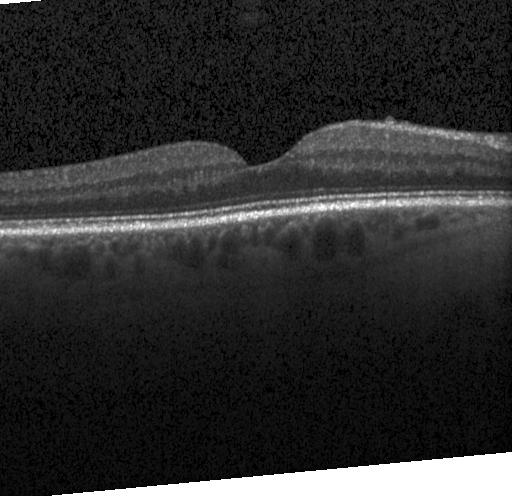 Spectral-domain optical coherence tomography · acquired on a Heidelberg Spectralis · retinal OCT B-scan. Impression: neither choroidal neovascularization, diabetic macular edema, nor drusen.